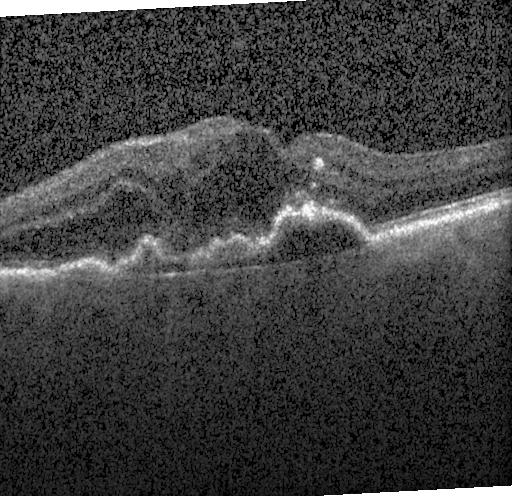

OCT line scan — Diagnosis: choroidal neovascularization.